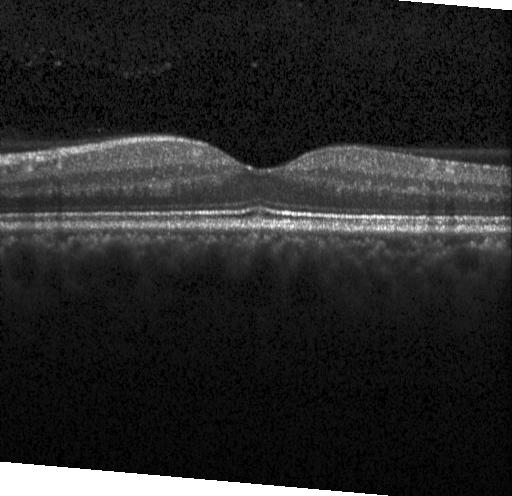 Macular OCT: neither choroidal neovascularization, diabetic macular edema, nor drusen.